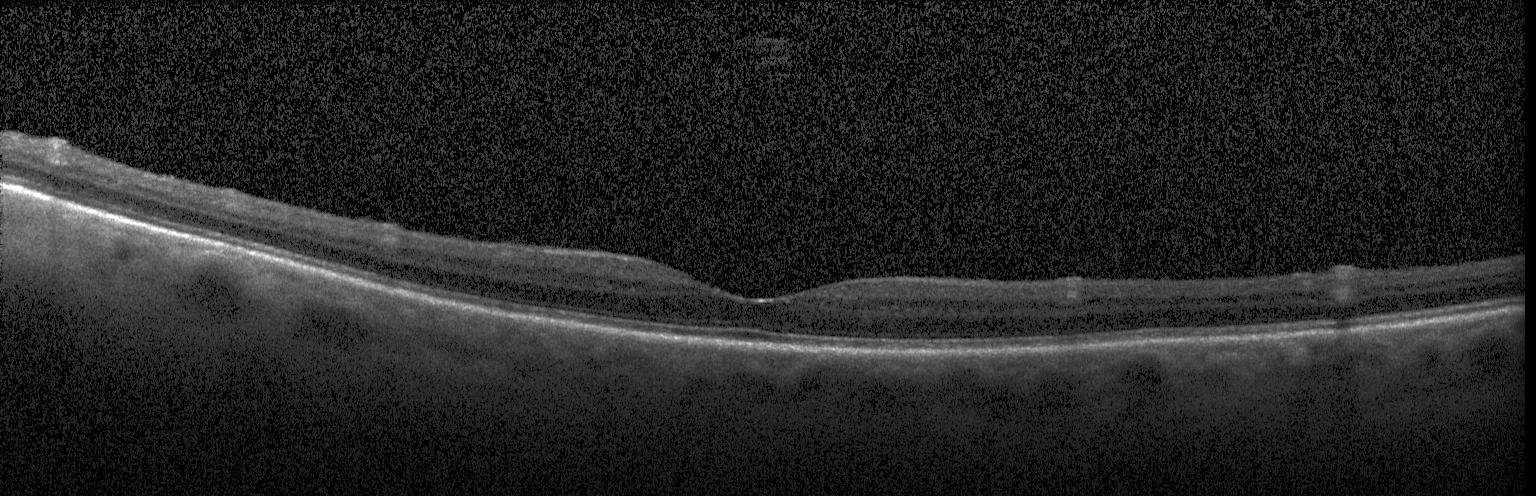

Optical coherence tomography B-scan · centered on the fovea · SD-OCT · Heidelberg Spectralis. Finding: no CNV, DME, or drusen.